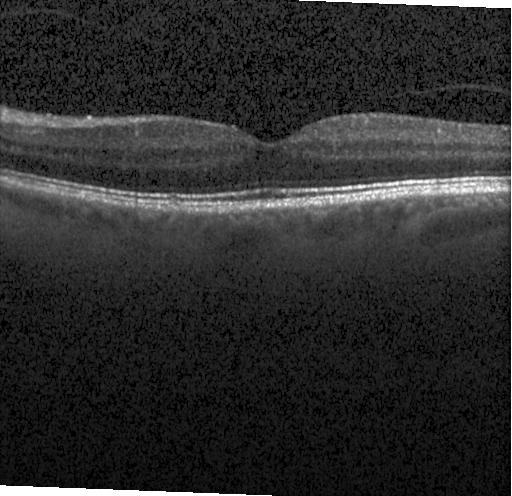

Optical coherence tomography scan. Diagnosis: no evidence of choroidal neovascularization, diabetic macular edema, or drusen.